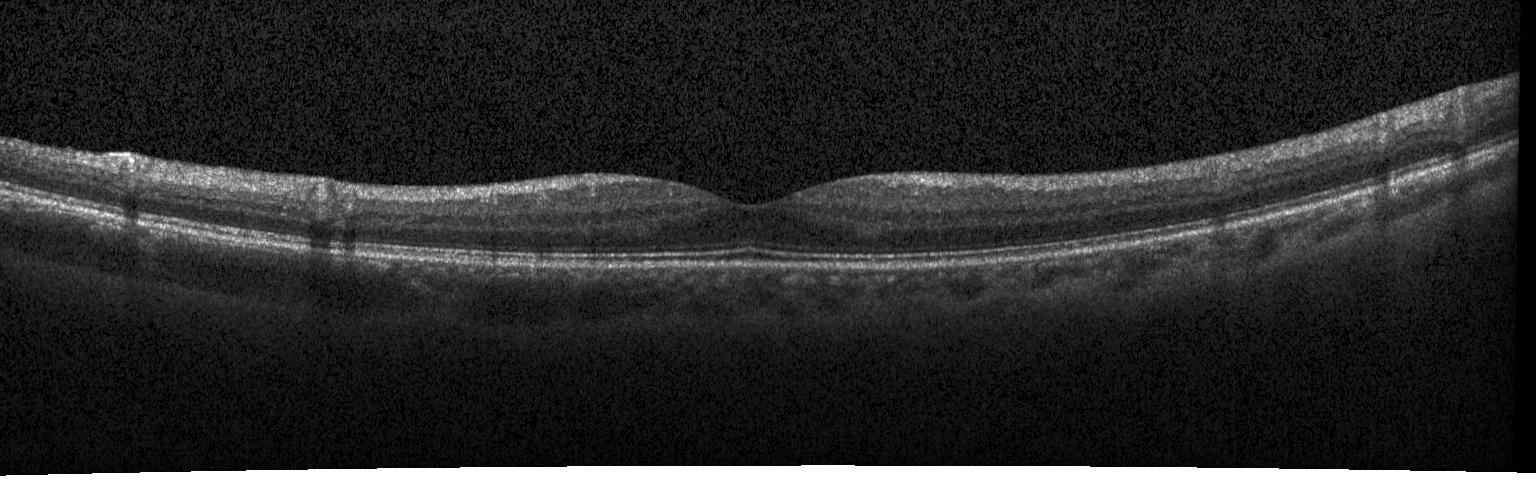

OCT scan showing no choroidal neovascularization, diabetic macular edema, or drusen.